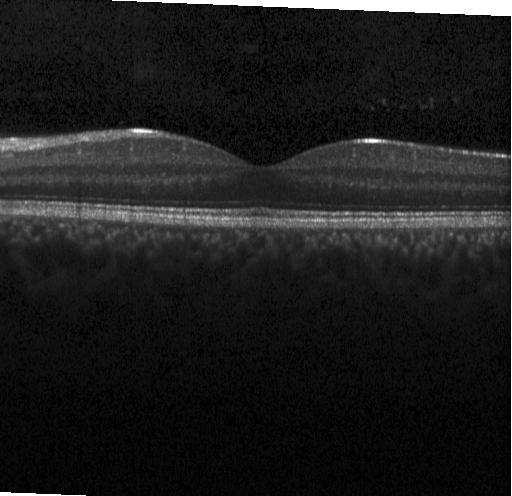

Retinal OCT cross-section; acquired on a Heidelberg Spectralis.
Diagnosis: neither CNV, DME, nor drusen.